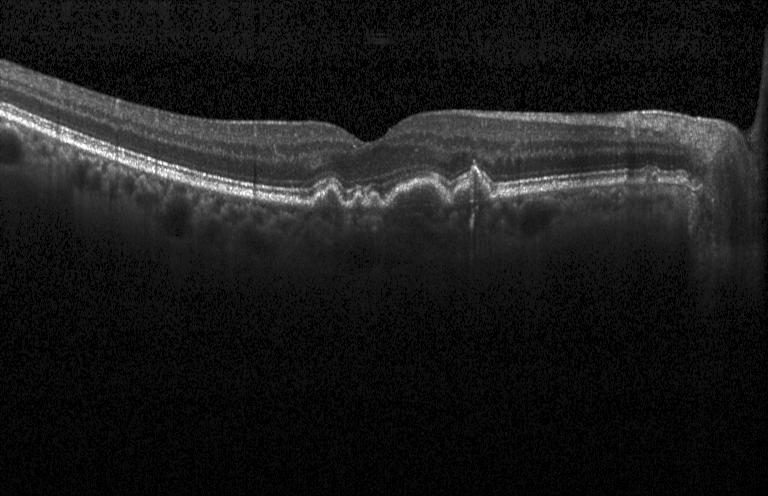
OCT finding: multiple drusen.